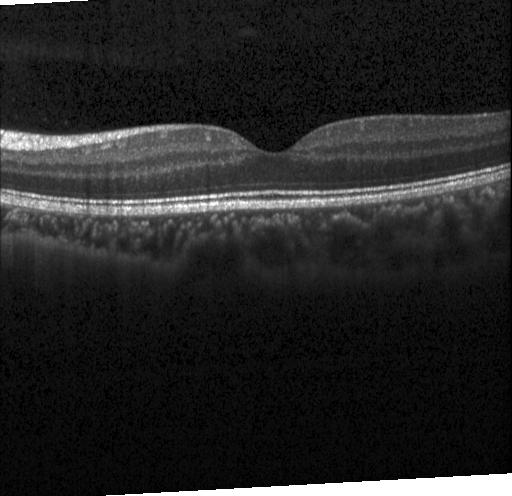

Spectral-domain OCT B-scan: no evidence of CNV, DME, or drusen.